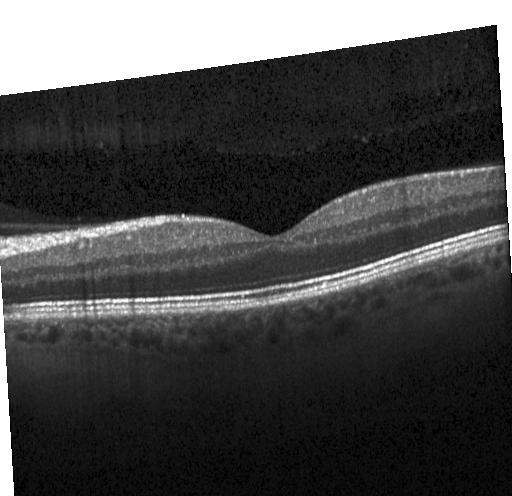
OCT line scan. Instrument: Heidelberg Spectralis.
The scan shows no CNV, no DME, and no drusen.